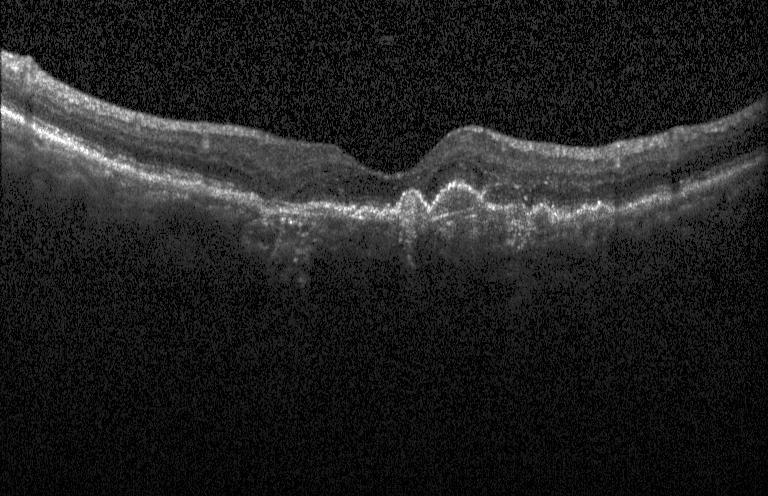 Retinal OCT cross-section. This B-scan demonstrates choroidal neovascularization.